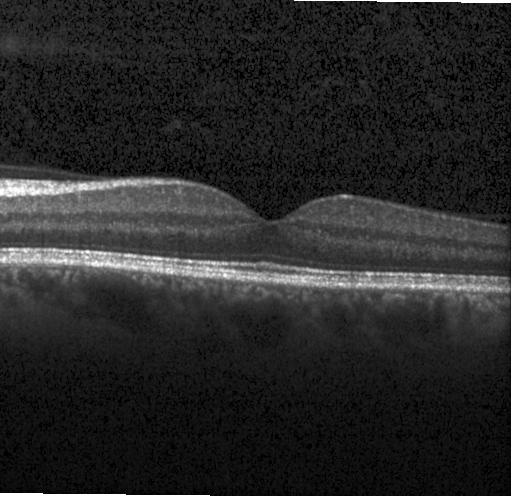 OCT B-scan
Macular OCT: no evidence of CNV, DME, or drusen.